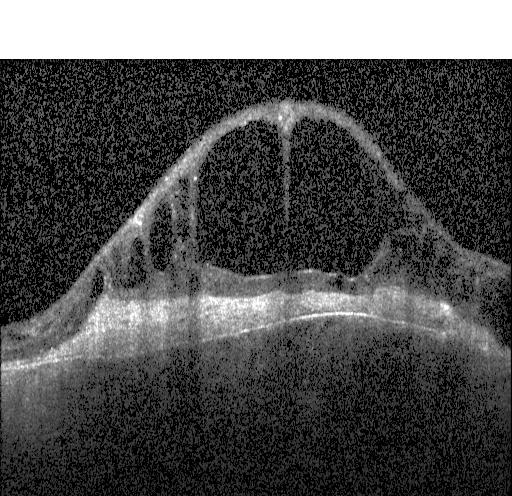
Retinal OCT B-scan; through the macula; instrument: Heidelberg Spectralis
Macular OCT: a choroidal neovascular membrane.